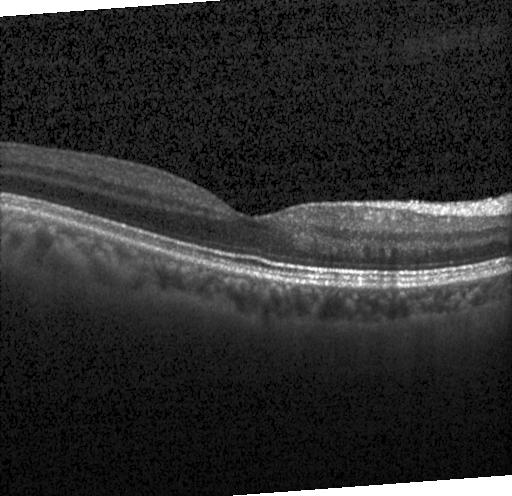

Instrument: Heidelberg Spectralis. Optical coherence tomography scan.
Impression: no CNV, no DME, and no drusen.